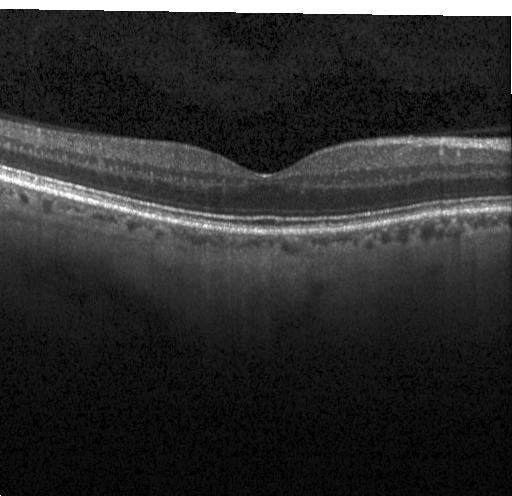
Retinal OCT cross-section, through the macula, Heidelberg Spectralis, SD-OCT — No choroidal neovascularization, diabetic macular edema, or drusen.